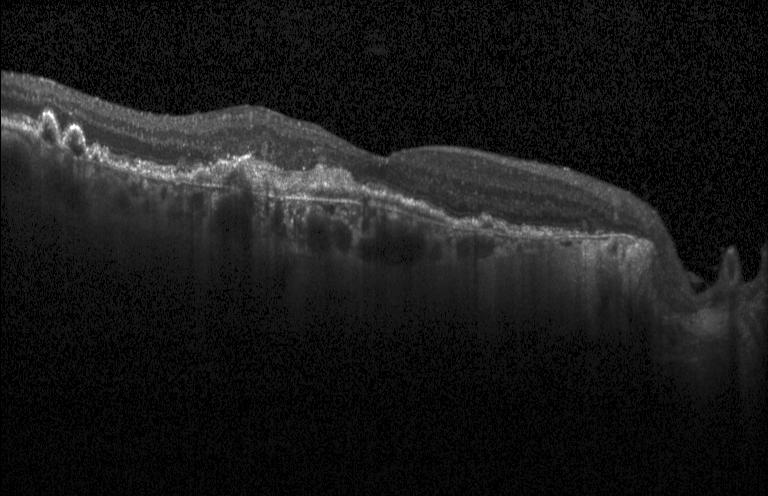
Finding: a choroidal neovascular membrane.